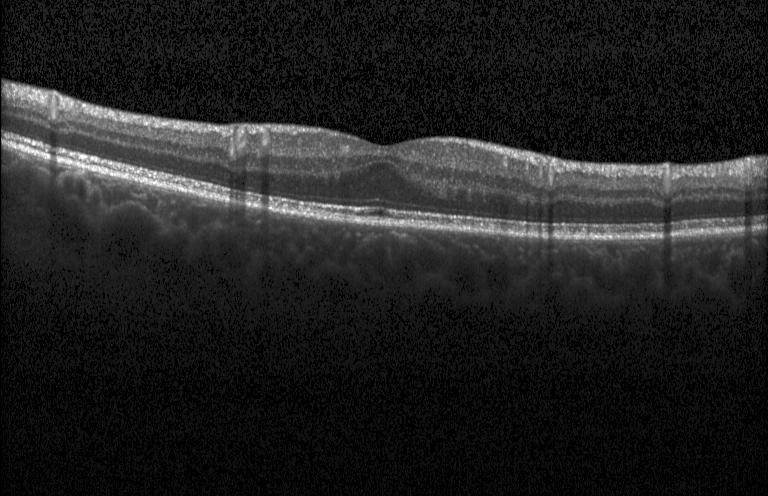

Retinal OCT cross-section showing no CNV, no DME, and no drusen.